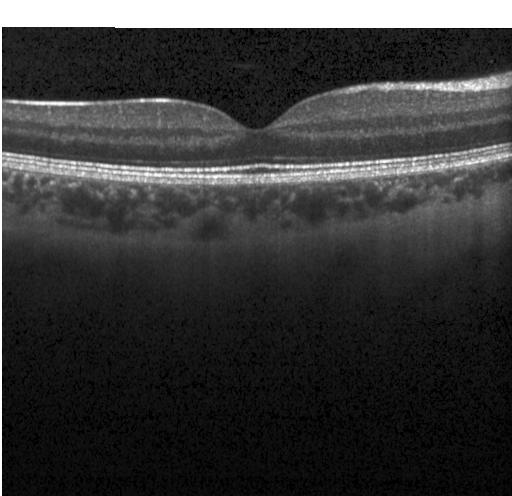
Retinal OCT cross-section — OCT finding: neither choroidal neovascularization, diabetic macular edema, nor drusen.